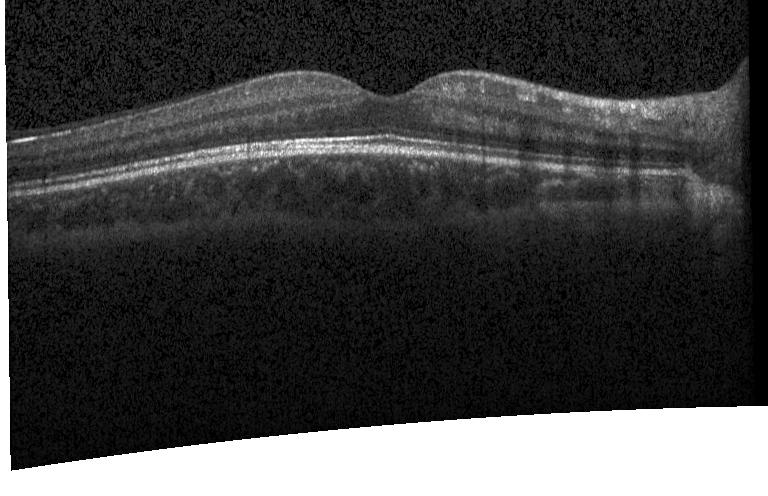
Spectral-domain OCT; Heidelberg Spectralis OCT system; optical coherence tomography scan — Impression: no evidence of choroidal neovascularization, diabetic macular edema, or drusen.